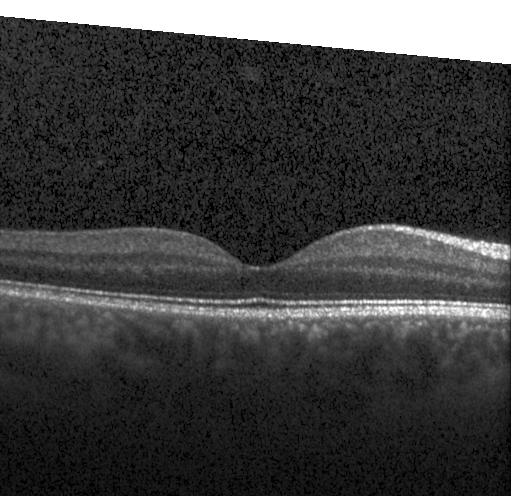

Retinal OCT B-scan. Heidelberg Spectralis OCT system. Macular scan. Spectral-domain optical coherence tomography.
Finding: neither choroidal neovascularization, diabetic macular edema, nor drusen.